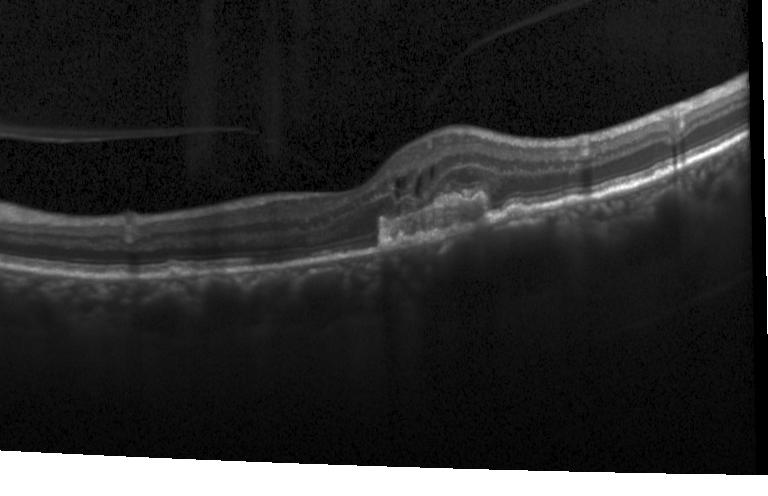

Macular OCT demonstrating a choroidal neovascular membrane.